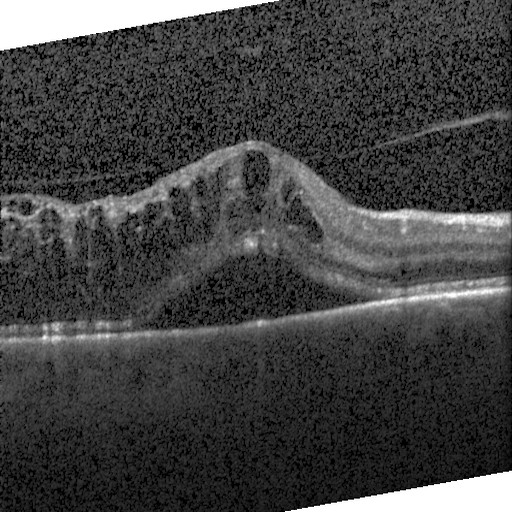
Retinal OCT B-scan. Fovea-centered. Spectral-domain OCT. Heidelberg Spectralis
Finding: diabetic macular edema.